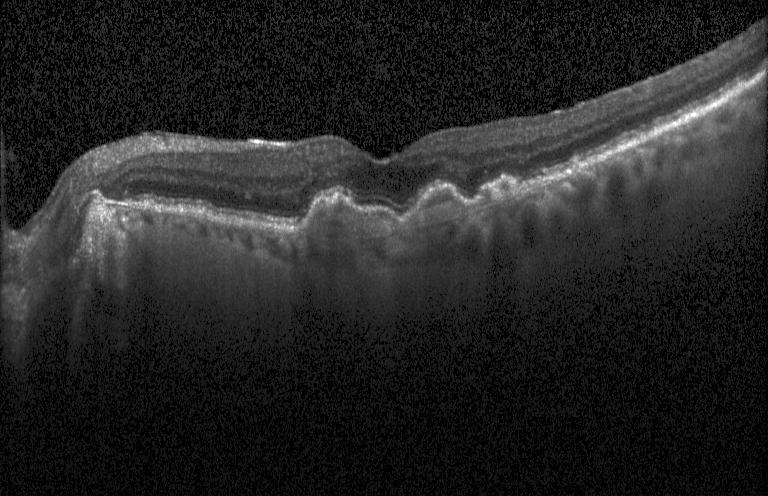 Finding: choroidal neovascularization.